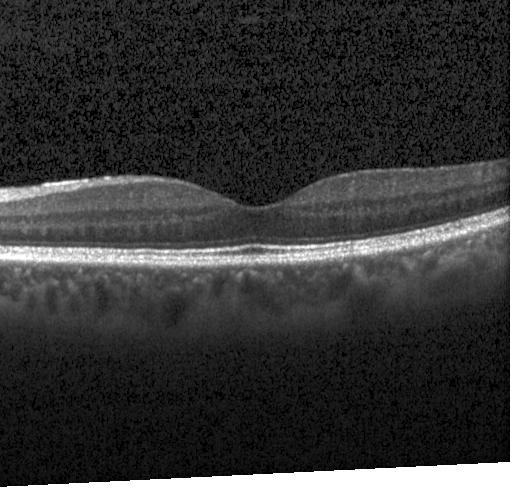
Dx: no evidence of choroidal neovascularization, diabetic macular edema, or drusen.